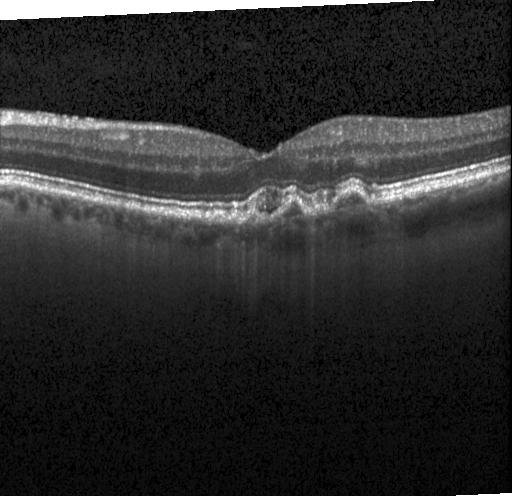

Optical coherence tomography B-scan — Finding: choroidal neovascularization.